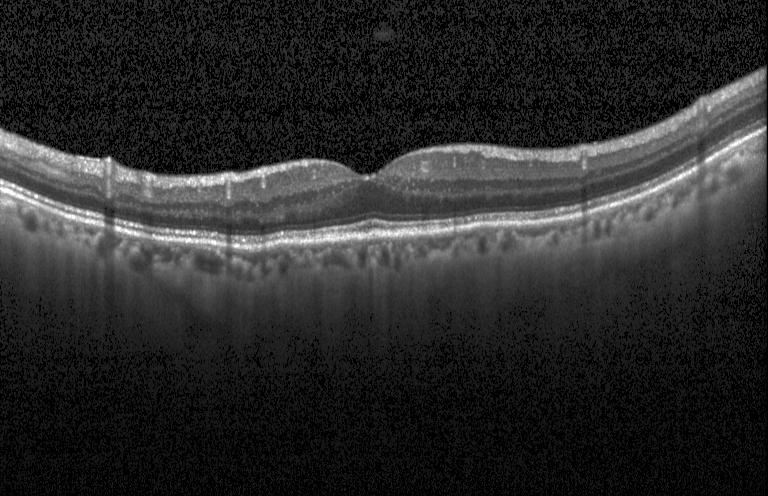

Centered on the fovea, OCT line scan, spectral-domain optical coherence tomography, Heidelberg Spectralis
Impression: no choroidal neovascularization, diabetic macular edema, or drusen.